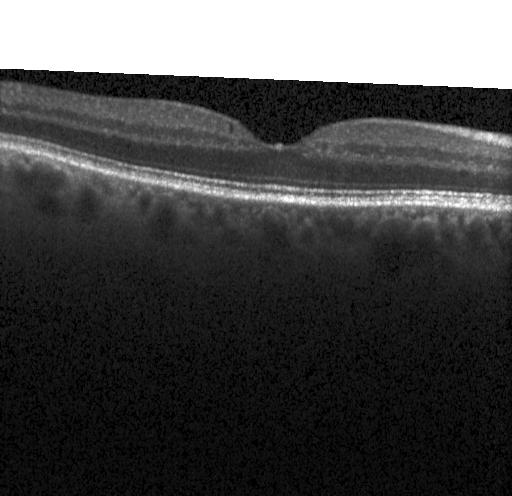 Macular scan, OCT line scan, spectral-domain OCT, acquired on a Heidelberg Spectralis — Finding: no evidence of choroidal neovascularization, diabetic macular edema, or drusen.